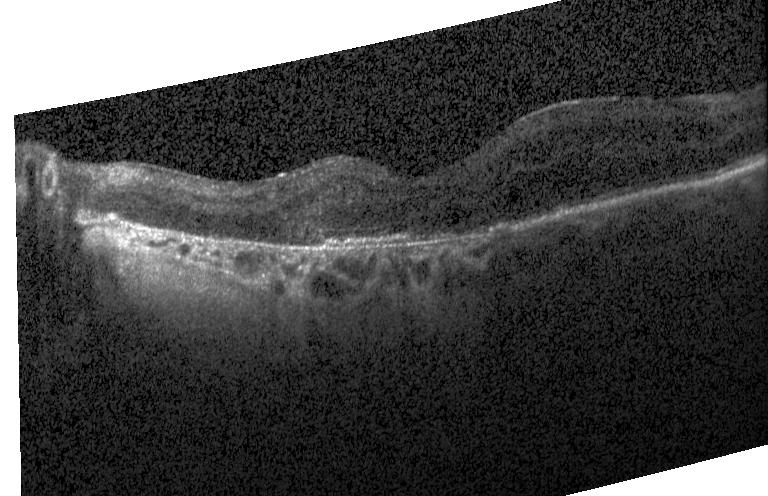 Fovea-centered; retinal OCT B-scan; instrument: Heidelberg Spectralis — The scan shows choroidal neovascularization.